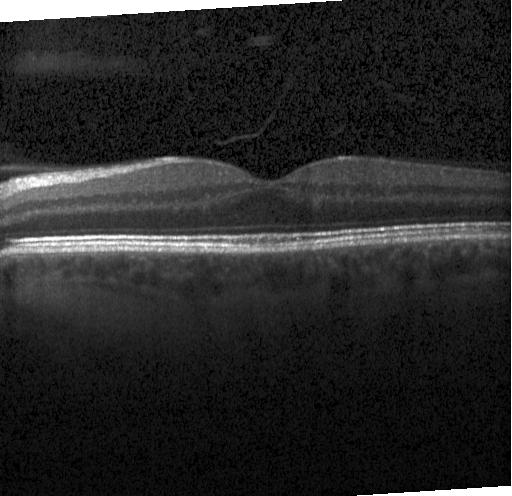
Retinal OCT B-scan.
Impression: no choroidal neovascularization, no diabetic macular edema, and no drusen.